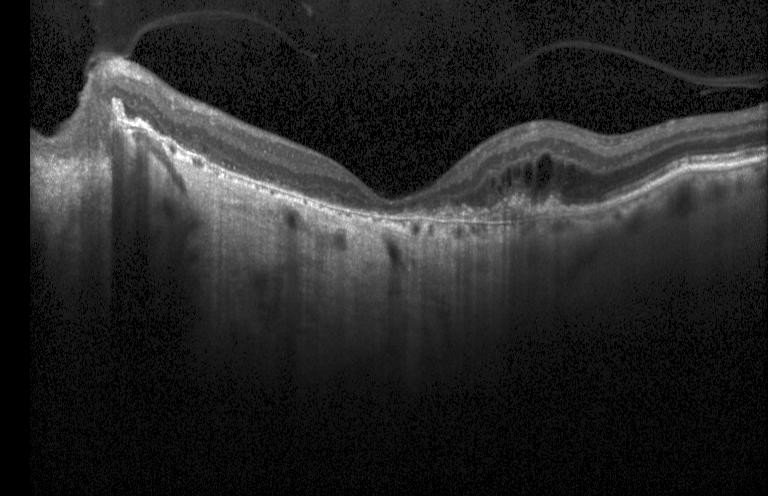

Heidelberg Spectralis OCT system. Spectral-domain optical coherence tomography. Macular scan. OCT line scan. Assessment: a choroidal neovascular membrane.